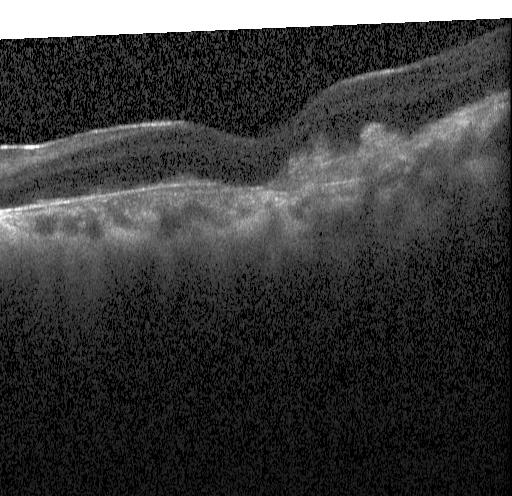
Retinal OCT B-scan.
The scan shows a choroidal neovascular membrane.